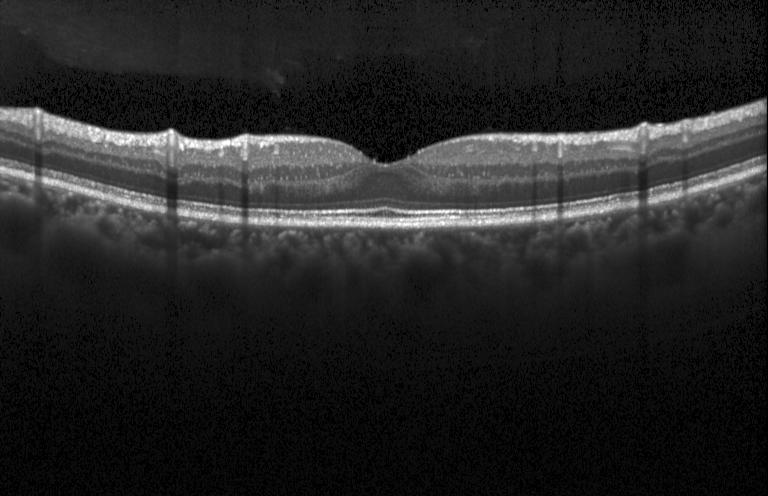 Fovea-centered; optical coherence tomography B-scan; Heidelberg Spectralis OCT system. Diagnosis: no choroidal neovascularization, diabetic macular edema, or drusen.